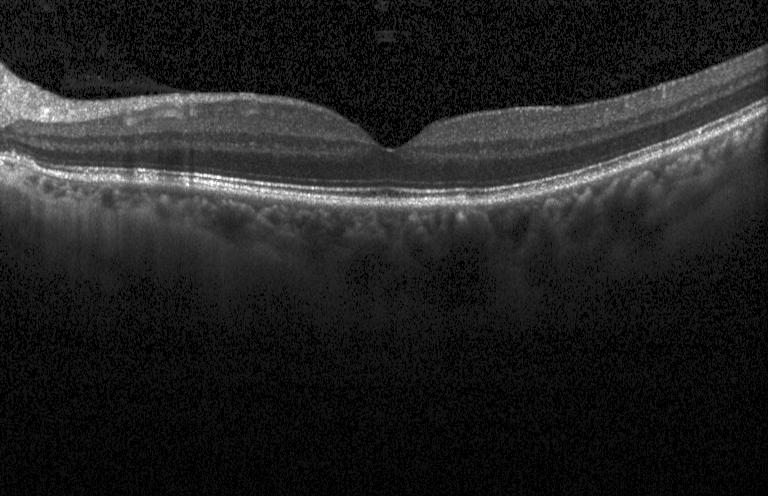
Optical coherence tomography B-scan.
OCT finding: neither choroidal neovascularization, diabetic macular edema, nor drusen.